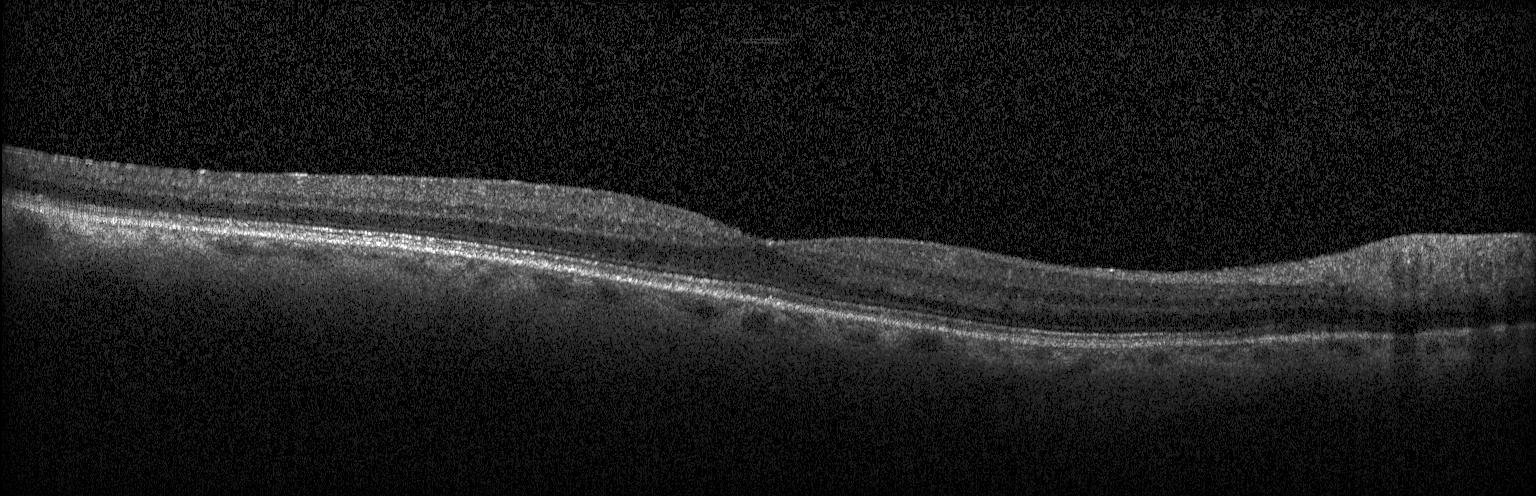 Macular scan, OCT line scan, instrument: Heidelberg Spectralis, spectral-domain OCT.
Finding: no evidence of choroidal neovascularization, diabetic macular edema, or drusen.